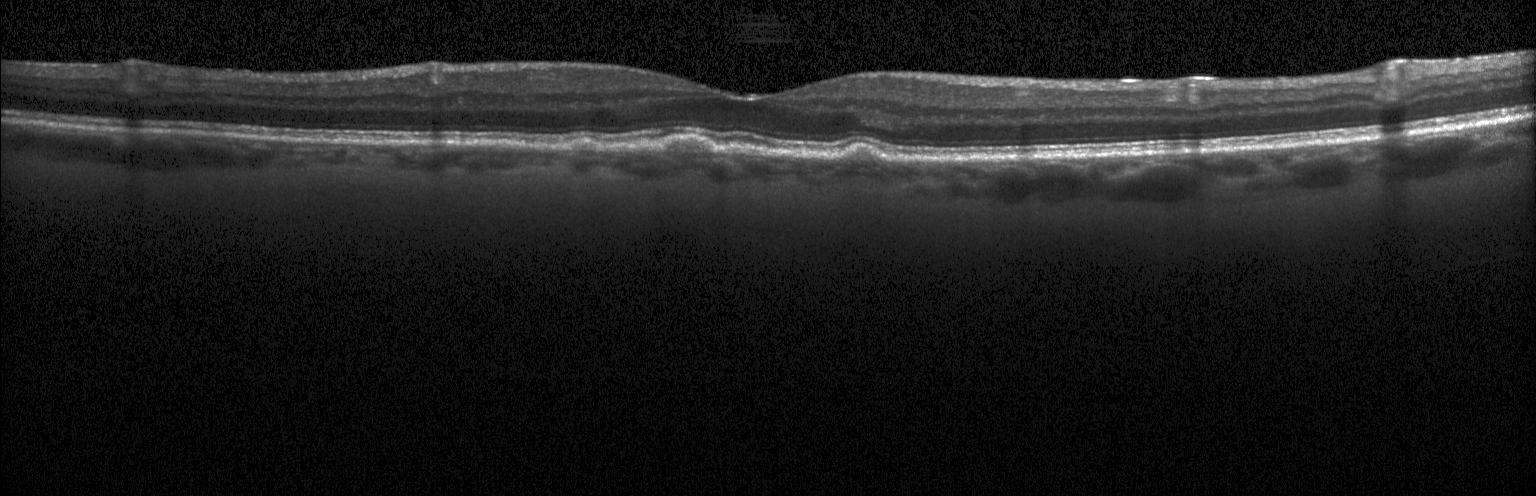
Optical coherence tomography B-scan · SD-OCT · Heidelberg Spectralis OCT system
Diagnosis: multiple drusen.